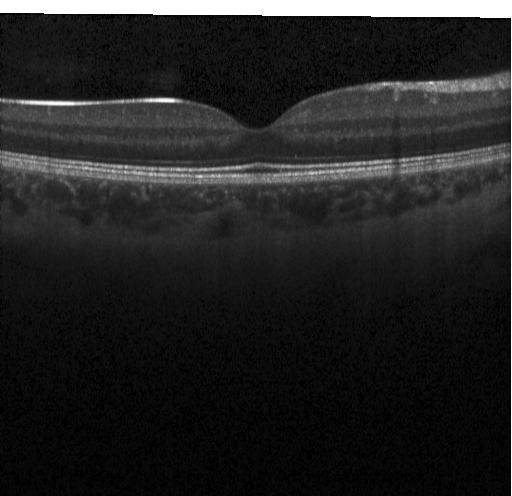

Spectral-domain optical coherence tomography, optical coherence tomography B-scan
Impression: no choroidal neovascularization, diabetic macular edema, or drusen.